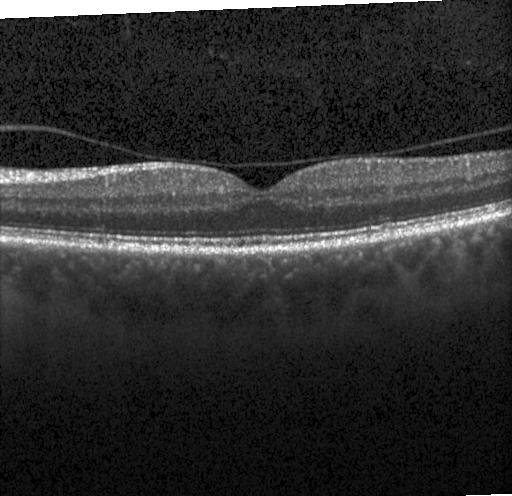 OCT finding: no choroidal neovascularization, diabetic macular edema, or drusen.